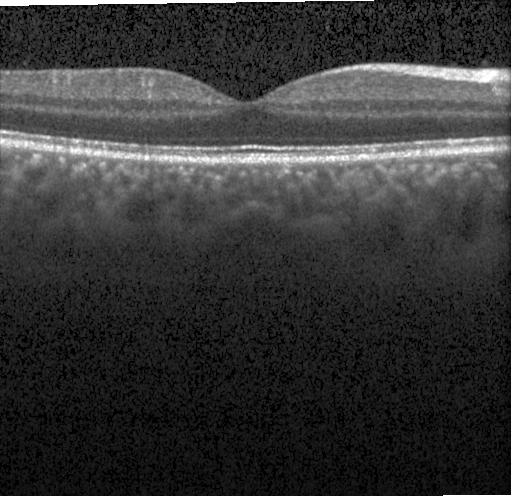

Heidelberg Spectralis, retinal OCT cross-section, fovea-centered. Diagnosis: neither CNV, DME, nor drusen.